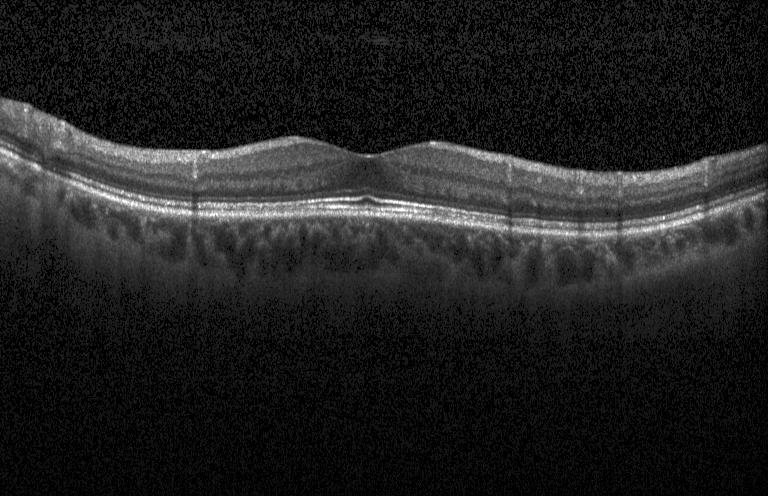 Assessment: no evidence of CNV, DME, or drusen.